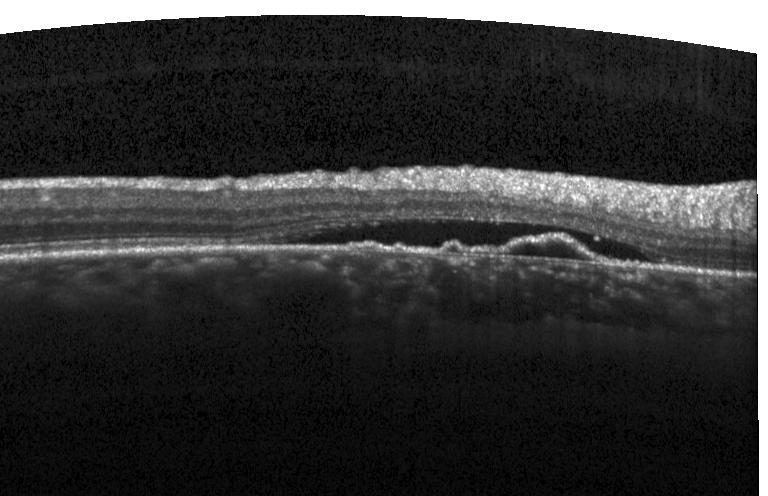

Spectral-domain OCT B-scan: a choroidal neovascular membrane.